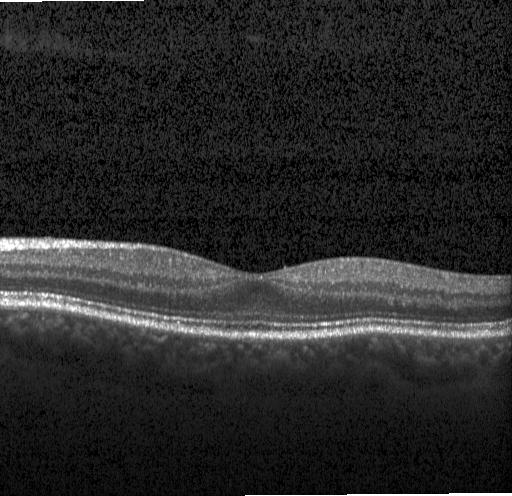 Optical coherence tomography B-scan
OCT finding: no evidence of CNV, DME, or drusen.